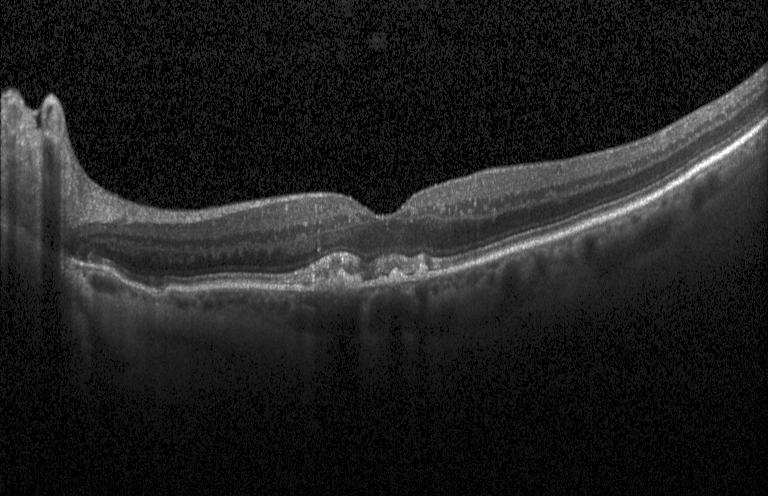
Horizontal scan through the fovea, optical coherence tomography B-scan — This B-scan demonstrates sub-RPE drusenoid deposits.